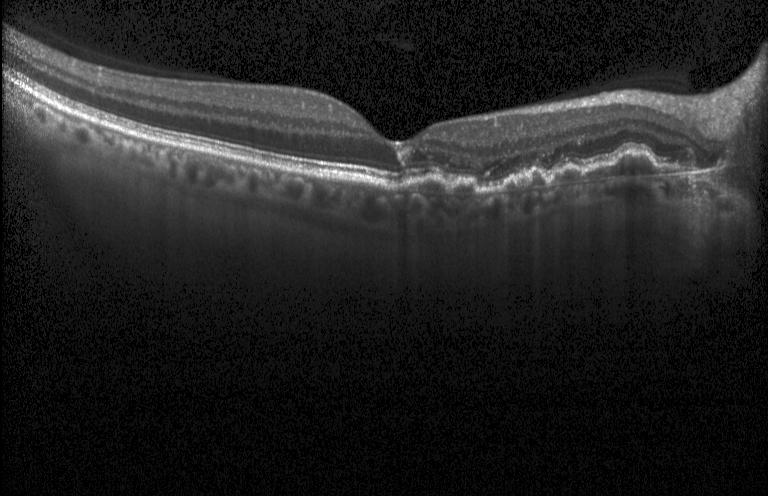

Optical coherence tomography scan
Impression: choroidal neovascularization (CNV).